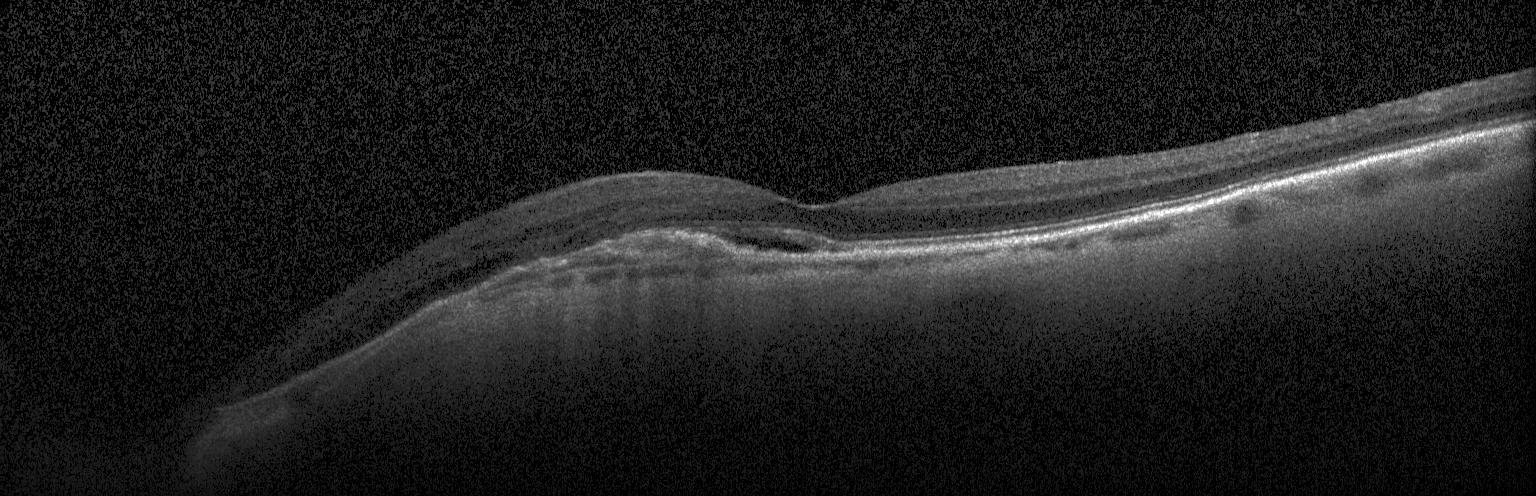 Finding: choroidal neovascularization.